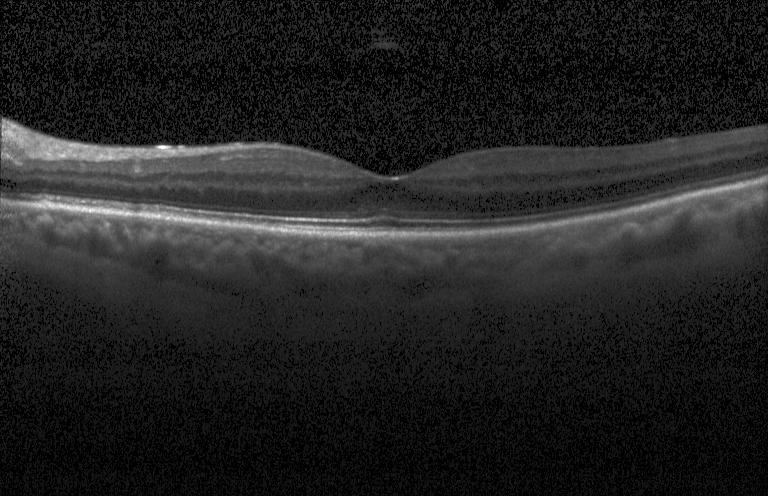 OCT line scan; SD-OCT
The scan shows no choroidal neovascularization, no diabetic macular edema, and no drusen.